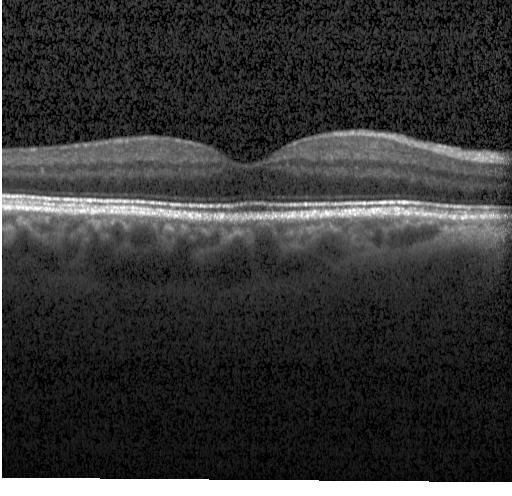 Horizontal scan through the fovea. SD-OCT. OCT B-scan
The scan shows no evidence of CNV, DME, or drusen.